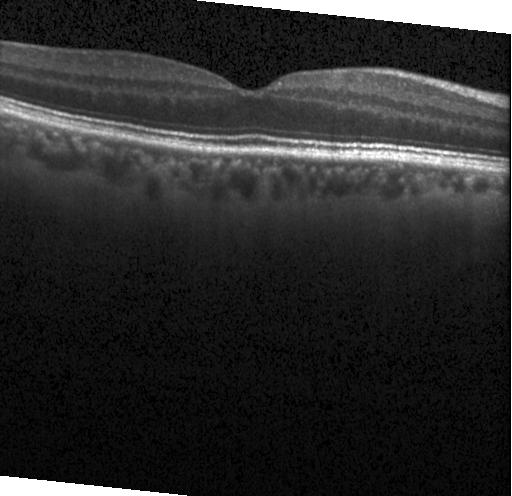

Retinal OCT cross-section
Impression: no choroidal neovascularization, no diabetic macular edema, and no drusen.